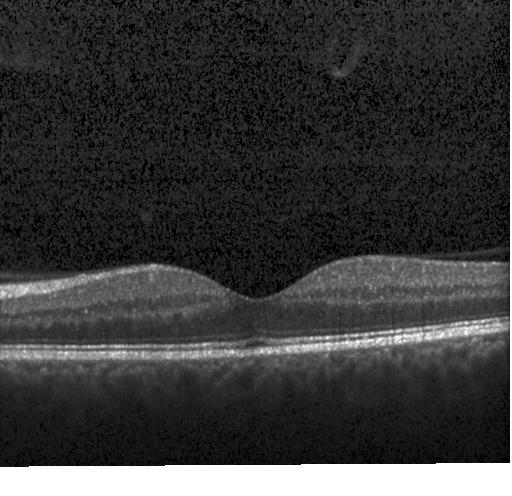 Instrument: Heidelberg Spectralis · optical coherence tomography scan. Neither choroidal neovascularization, diabetic macular edema, nor drusen.